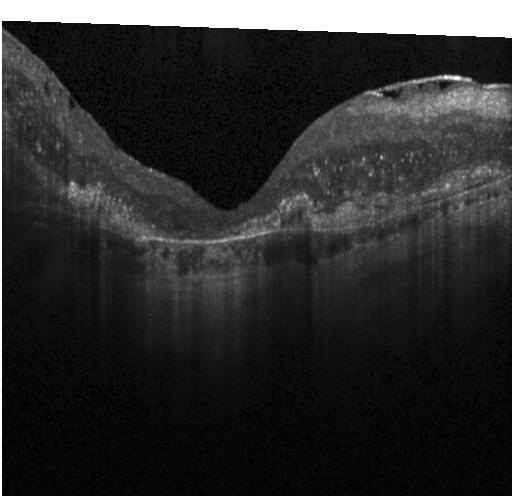 Instrument: Heidelberg Spectralis, optical coherence tomography B-scan
Impression: a choroidal neovascular membrane.